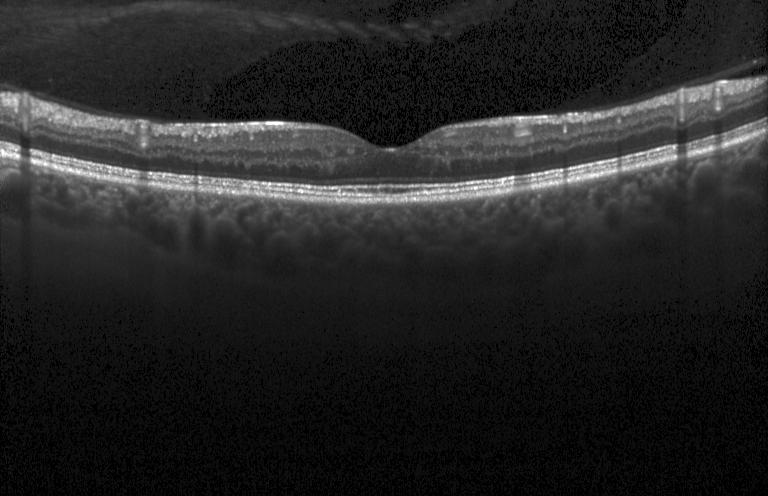

OCT line scan — OCT finding: no choroidal neovascularization, diabetic macular edema, or drusen.